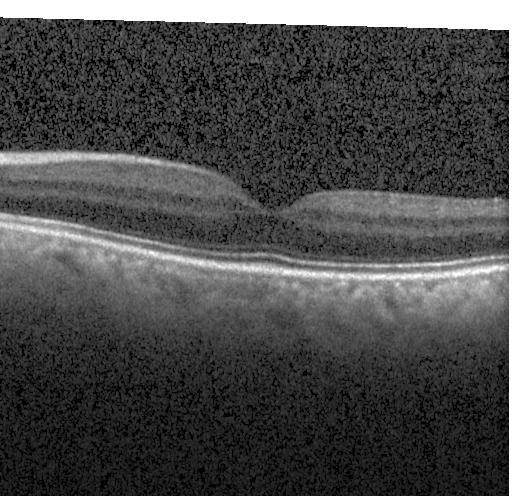
Diagnosis: no evidence of choroidal neovascularization, diabetic macular edema, or drusen.